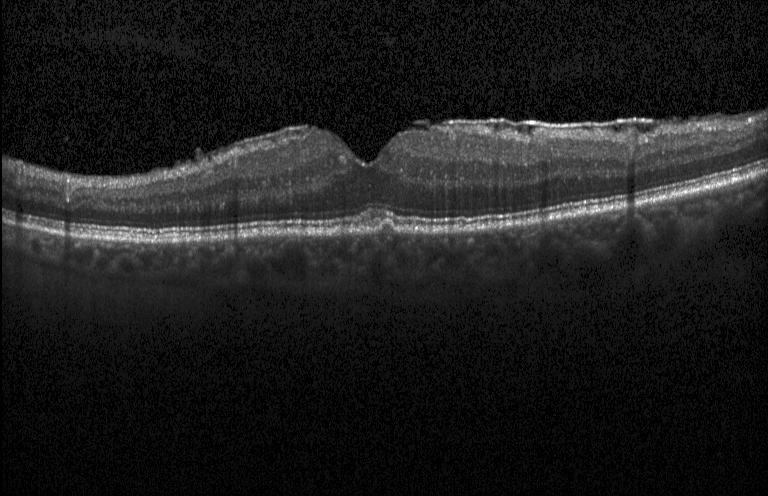
Spectral-domain optical coherence tomography. Acquired on a Heidelberg Spectralis. OCT B-scan. Through the macula. Impression: sub-RPE drusenoid deposits.